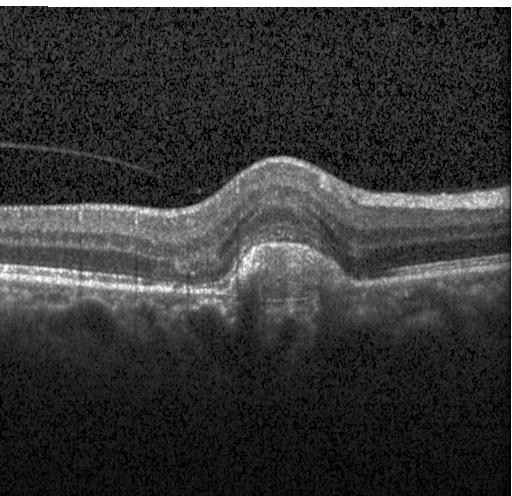

Optical coherence tomography scan.
Assessment: choroidal neovascularization.